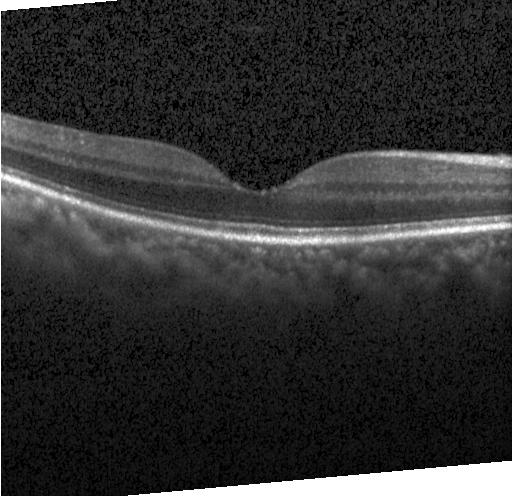
Finding: neither CNV, DME, nor drusen.